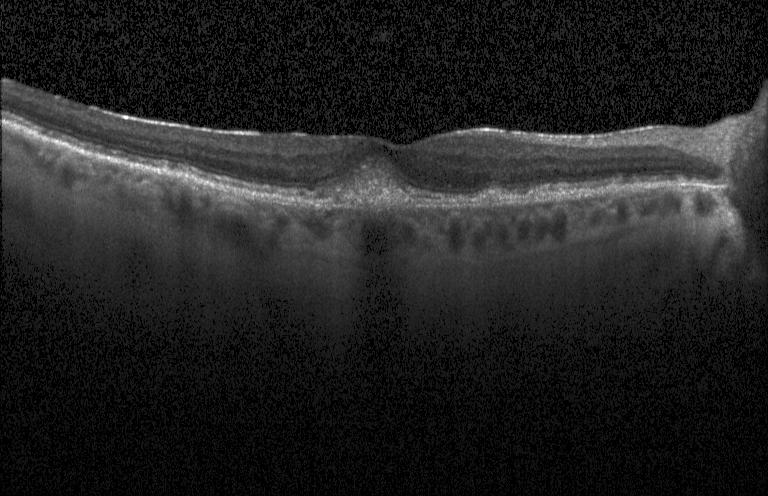

Centered on the fovea; optical coherence tomography B-scan.
Assessment: choroidal neovascularization.